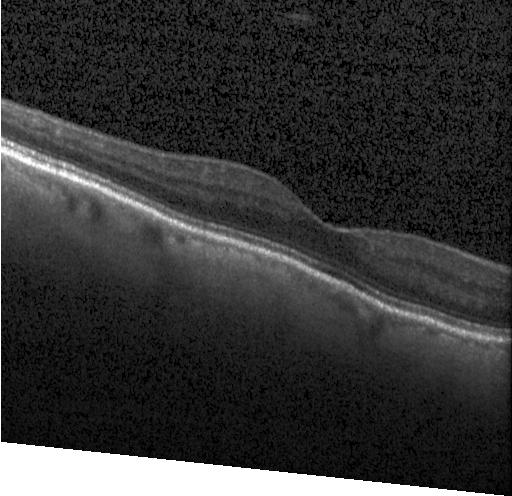 Instrument: Heidelberg Spectralis. OCT B-scan
OCT finding: neither choroidal neovascularization, diabetic macular edema, nor drusen.